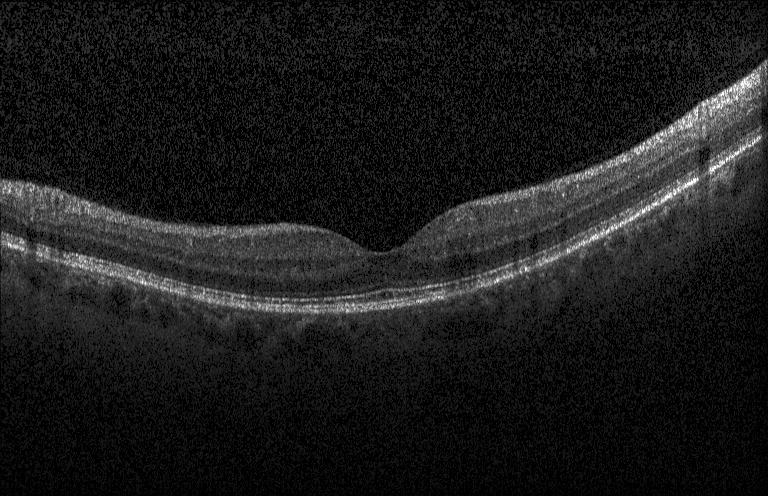
Retinal OCT B-scan — Assessment: neither CNV, DME, nor drusen.